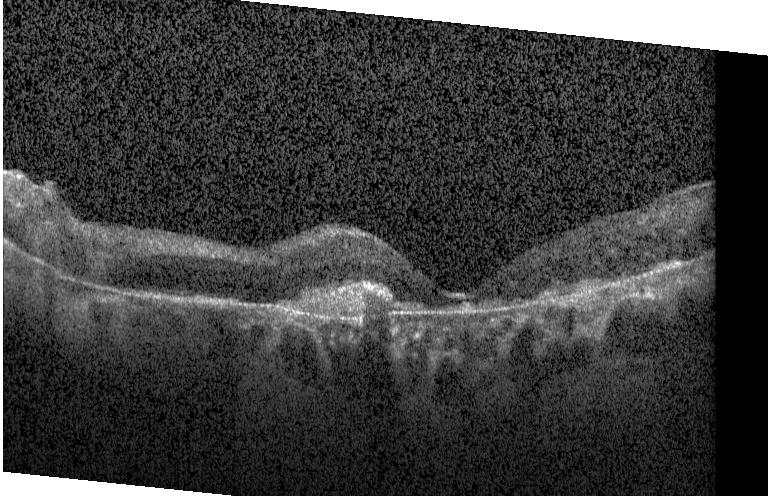

OCT scan showing a choroidal neovascular membrane.